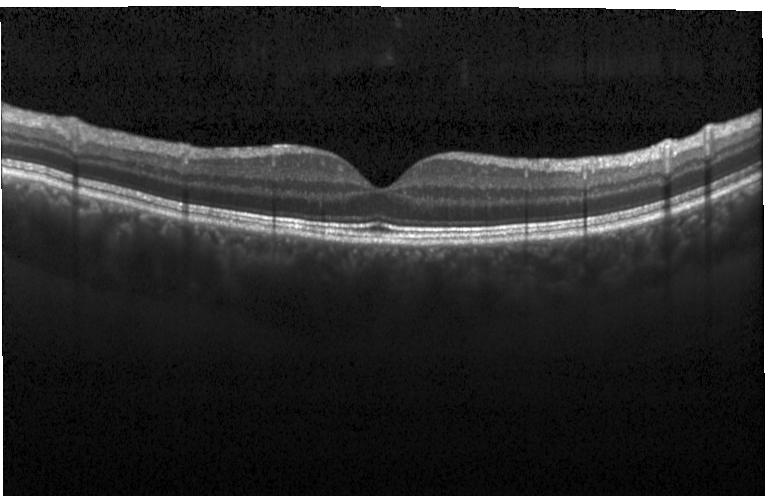
Optical coherence tomography scan · through the macula. Macular OCT: no evidence of CNV, DME, or drusen.